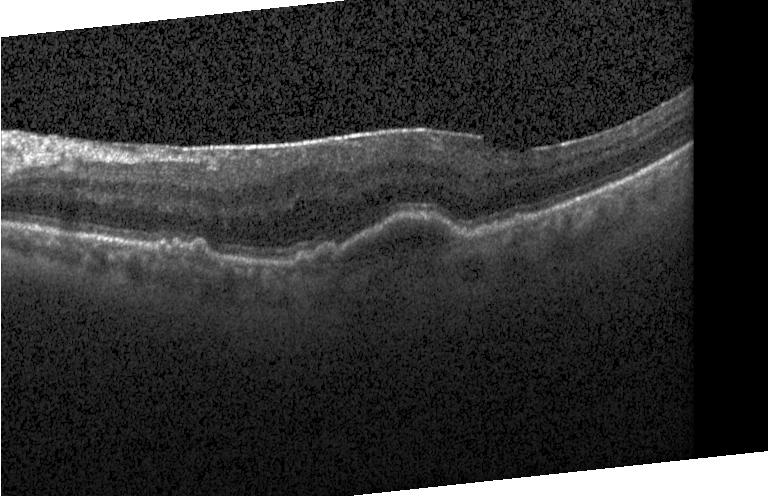 Finding: CNV.